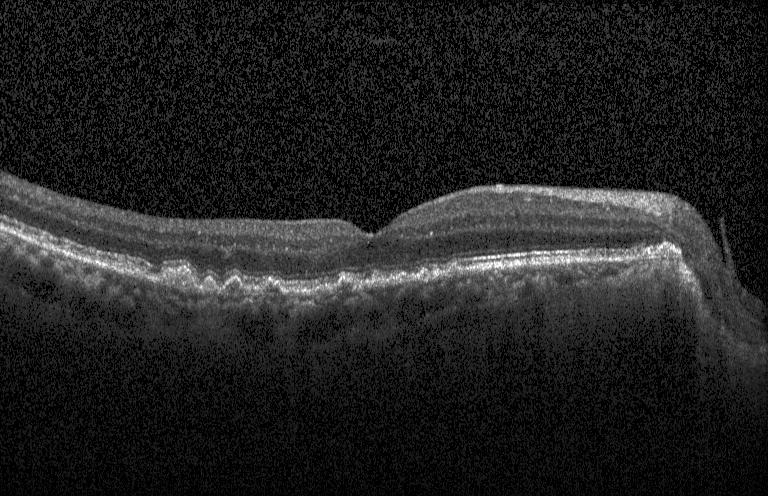

Macular OCT: multiple drusen.